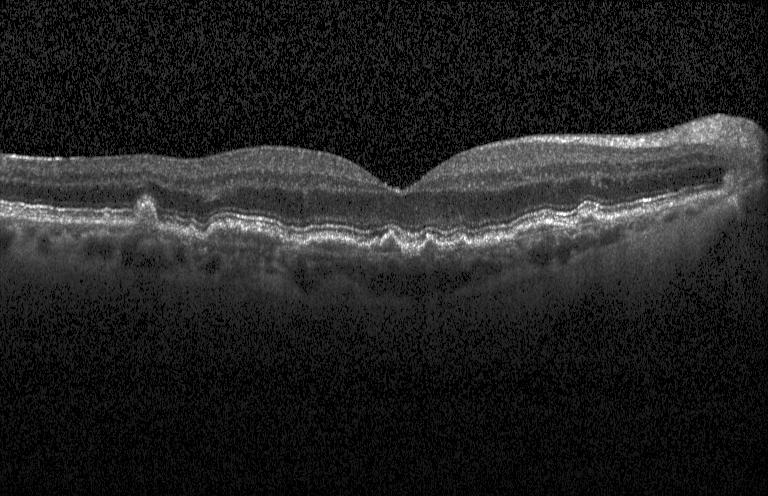 Heidelberg Spectralis, through the macula, spectral-domain optical coherence tomography, retinal OCT B-scan — Impression: multiple drusen.